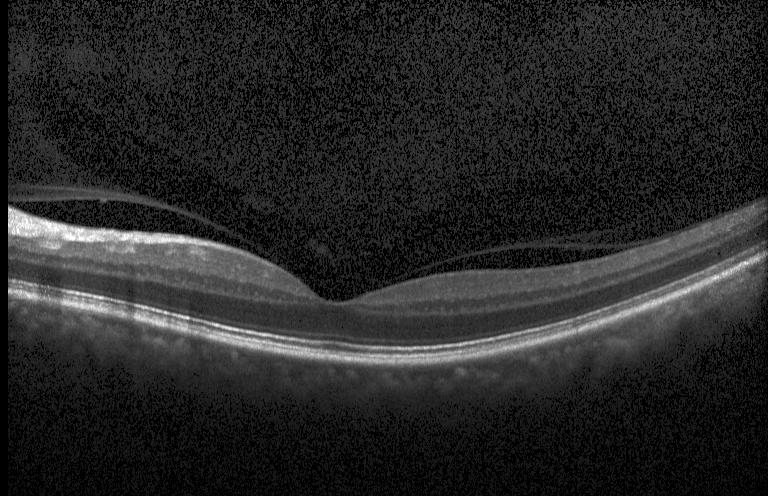
Retinal OCT B-scan.
Assessment: no CNV, DME, or drusen.